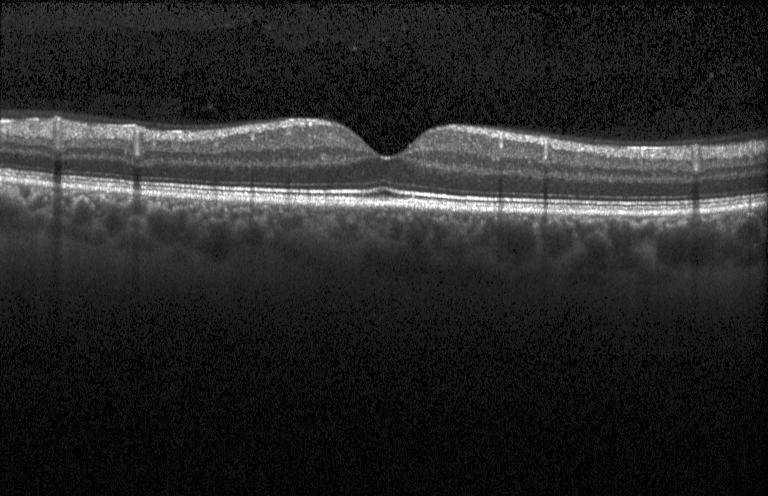
Finding: no evidence of CNV, DME, or drusen.